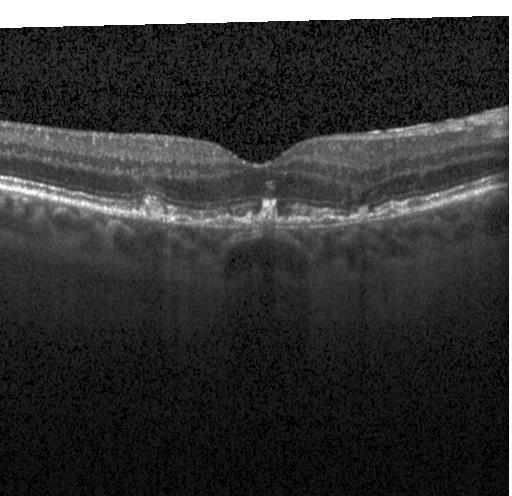
The scan shows choroidal neovascularization.